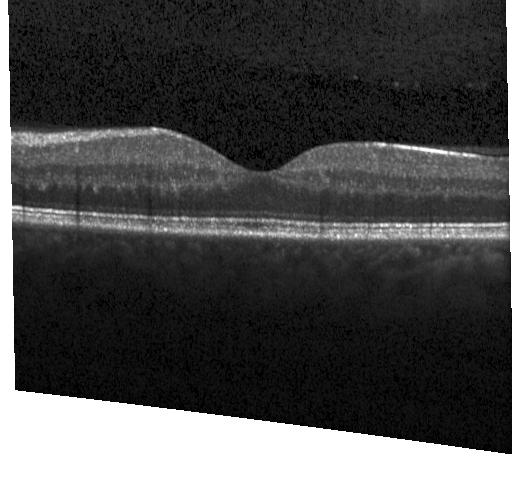

OCT B-scan
Assessment: no choroidal neovascularization, no diabetic macular edema, and no drusen.